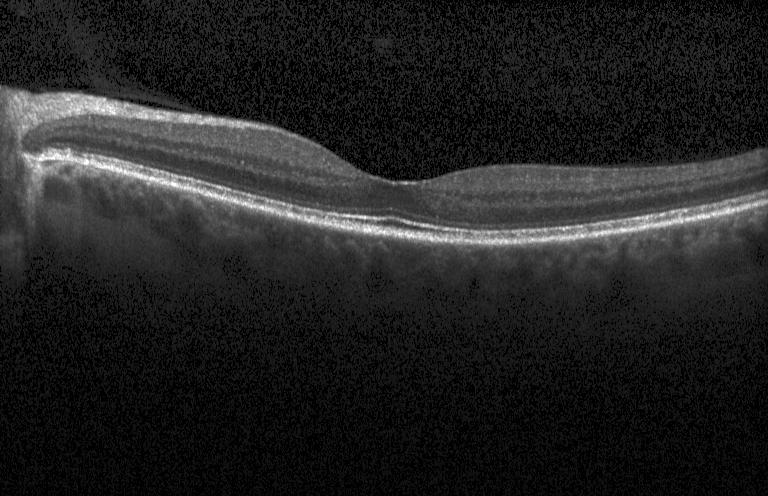 Optical coherence tomography scan, spectral-domain OCT
This B-scan demonstrates no choroidal neovascularization, diabetic macular edema, or drusen.